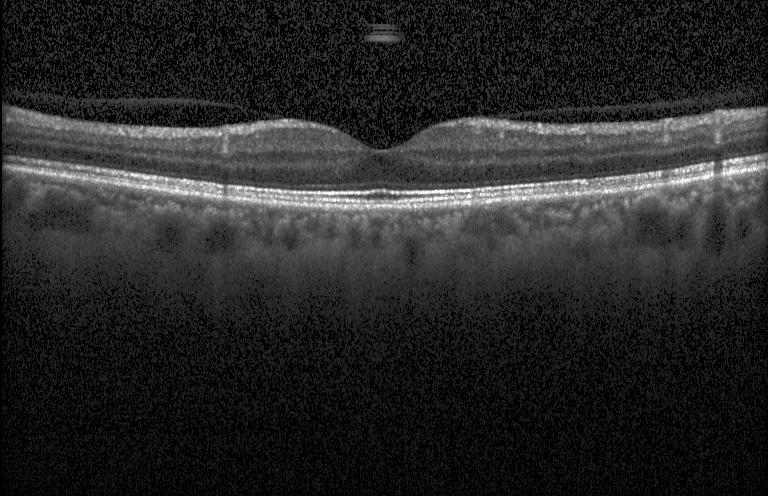
Macular OCT demonstrating no choroidal neovascularization, diabetic macular edema, or drusen.